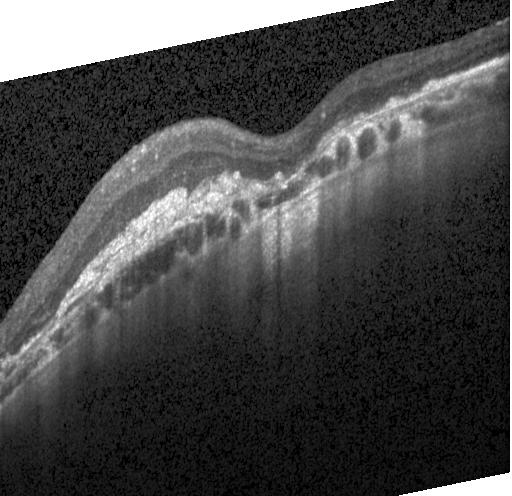 Through the macula, optical coherence tomography scan, acquired on a Heidelberg Spectralis.
Diagnosis: a choroidal neovascular membrane.